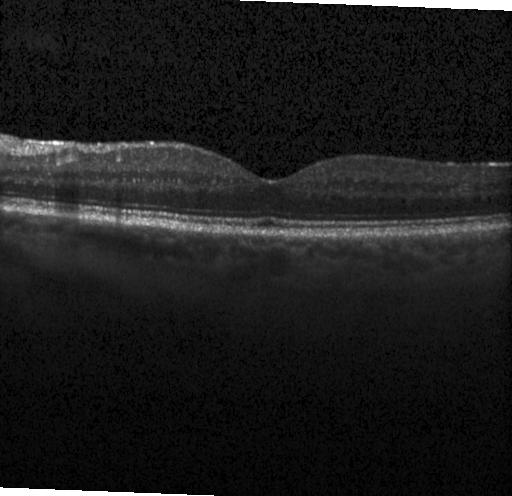 Dx: no evidence of CNV, DME, or drusen.